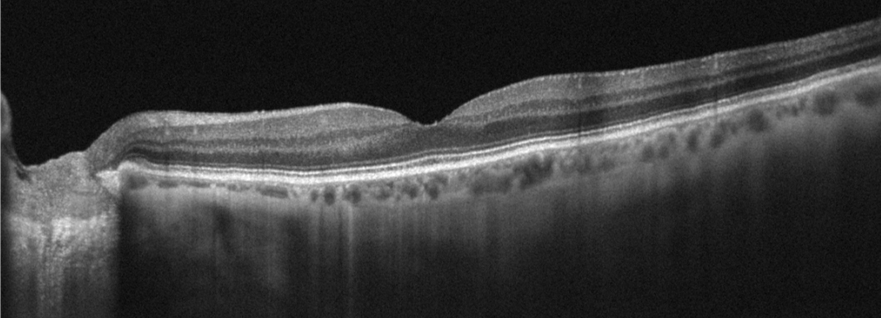
Macular scan. Acquired on an Optovue Avanti RTVue XR. OCT B-scan. OCT finding: AMD.